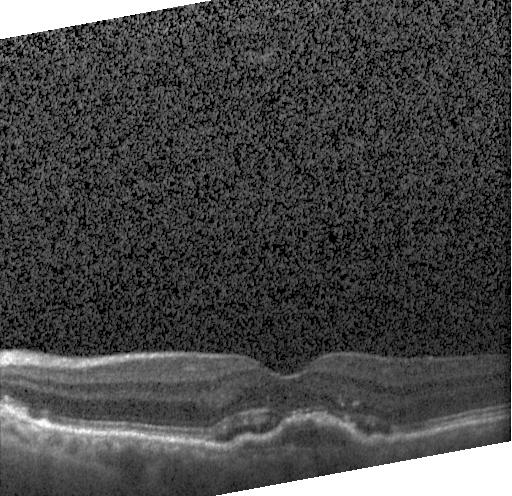 Diagnosis: choroidal neovascularization (CNV).